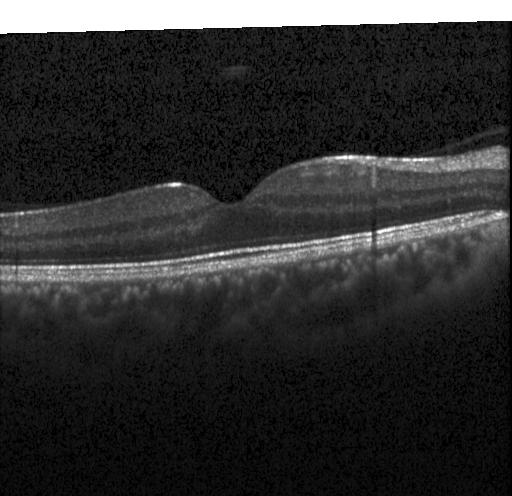 Heidelberg Spectralis. OCT line scan. Spectral-domain OCT.
OCT finding: no choroidal neovascularization, no diabetic macular edema, and no drusen.